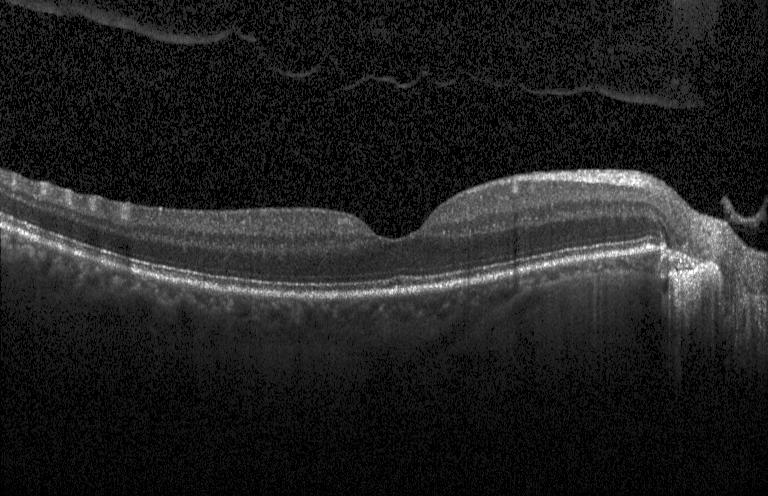
Finding: no choroidal neovascularization, no diabetic macular edema, and no drusen.